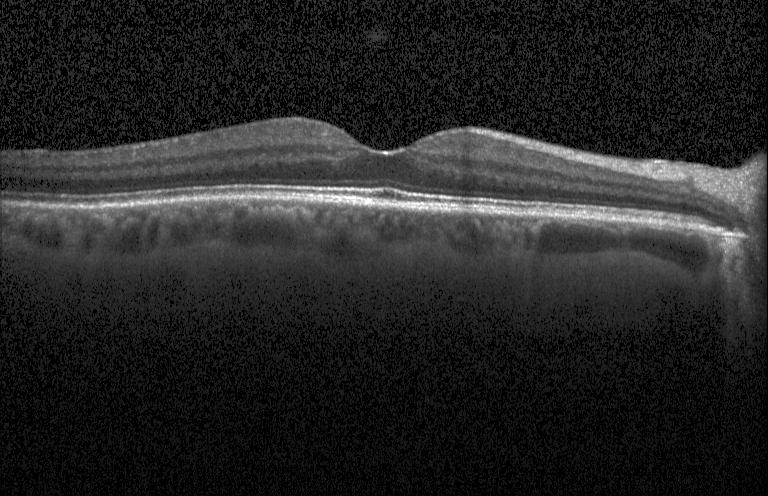

Retinal OCT B-scan, Heidelberg Spectralis
The scan shows no evidence of choroidal neovascularization, diabetic macular edema, or drusen.